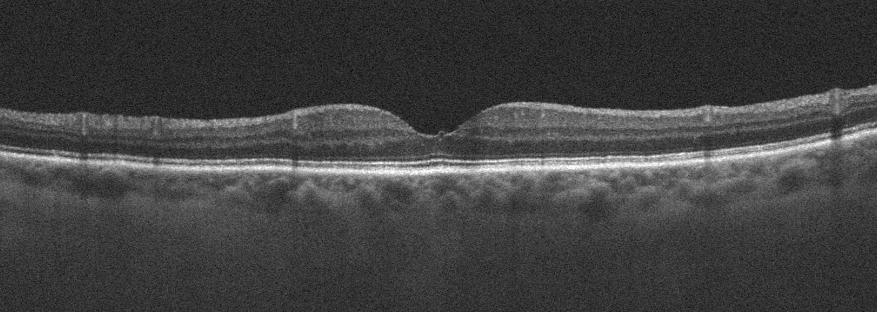

Instrument: Optovue Avanti RTVue XR. Retinal OCT cross-section. Fovea-centered. Impression: absence of AMD, DME, ERM, RAO, RVO, and vitreomacular interface disease.